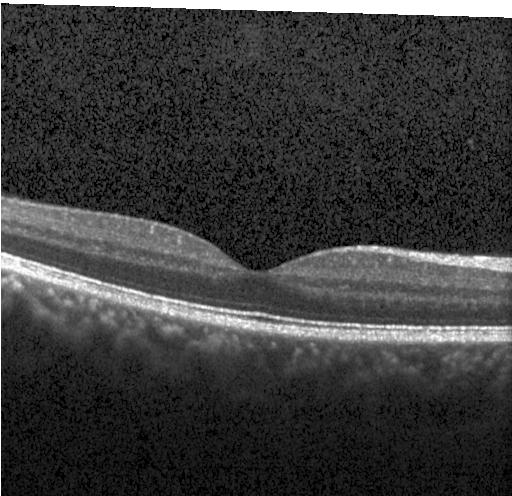
Dx: no evidence of choroidal neovascularization, diabetic macular edema, or drusen.